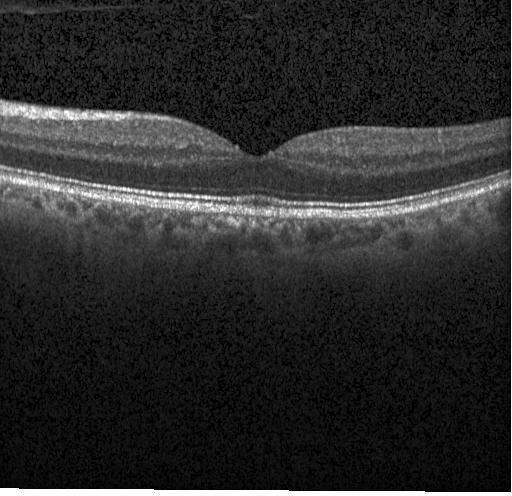
SD-OCT; retinal OCT B-scan.
Diagnosis: neither CNV, DME, nor drusen.